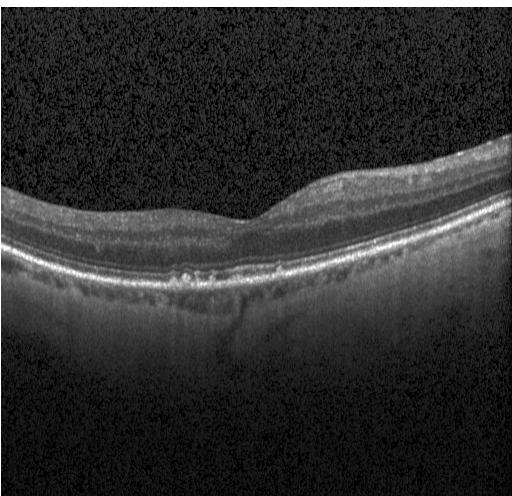 OCT scan showing multiple drusen.